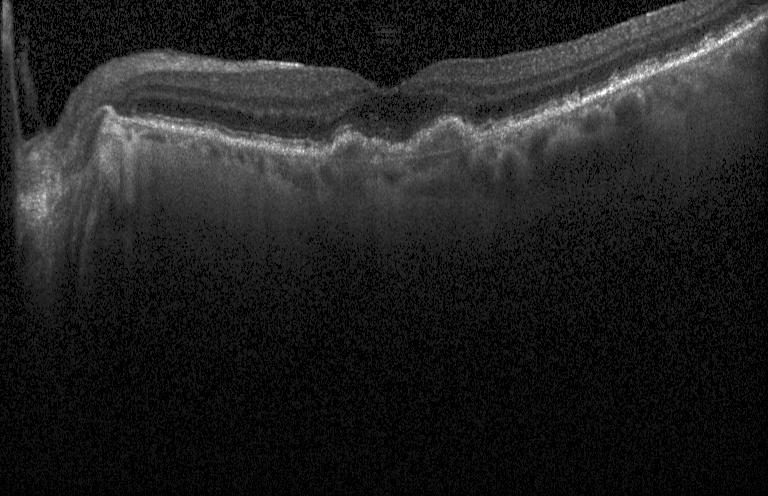

Optical coherence tomography B-scan — A choroidal neovascular membrane.